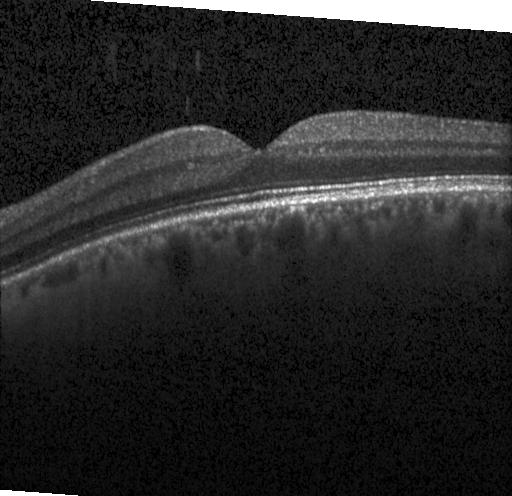 Impression: no evidence of choroidal neovascularization, diabetic macular edema, or drusen.